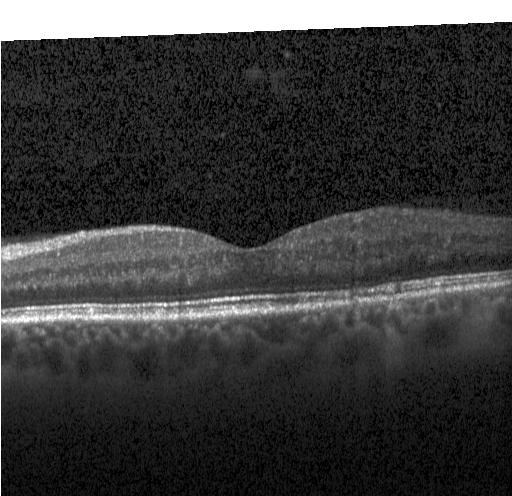
Impression: no choroidal neovascularization, diabetic macular edema, or drusen.